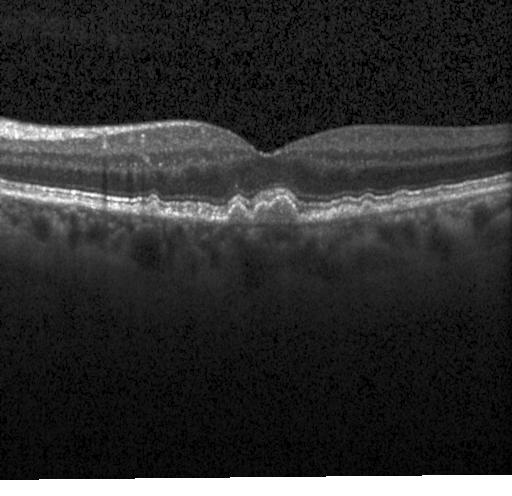
OCT B-scan.
The scan shows sub-RPE drusenoid deposits.